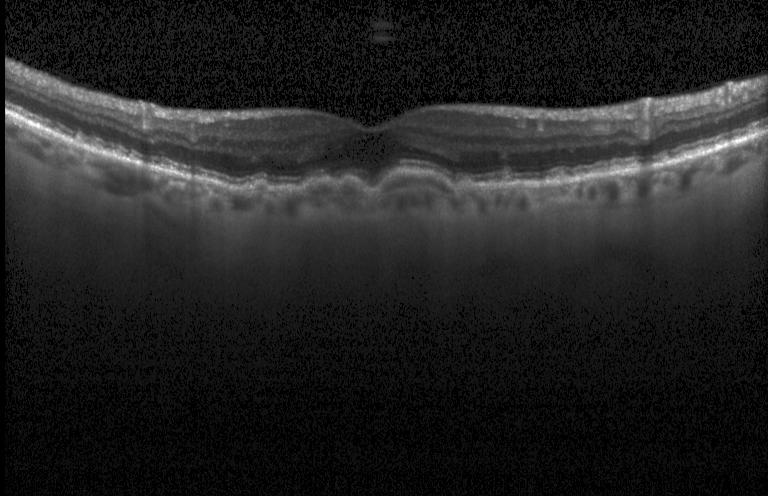

Optical coherence tomography scan · spectral-domain optical coherence tomography · acquired on a Heidelberg Spectralis · fovea-centered — Drusen.